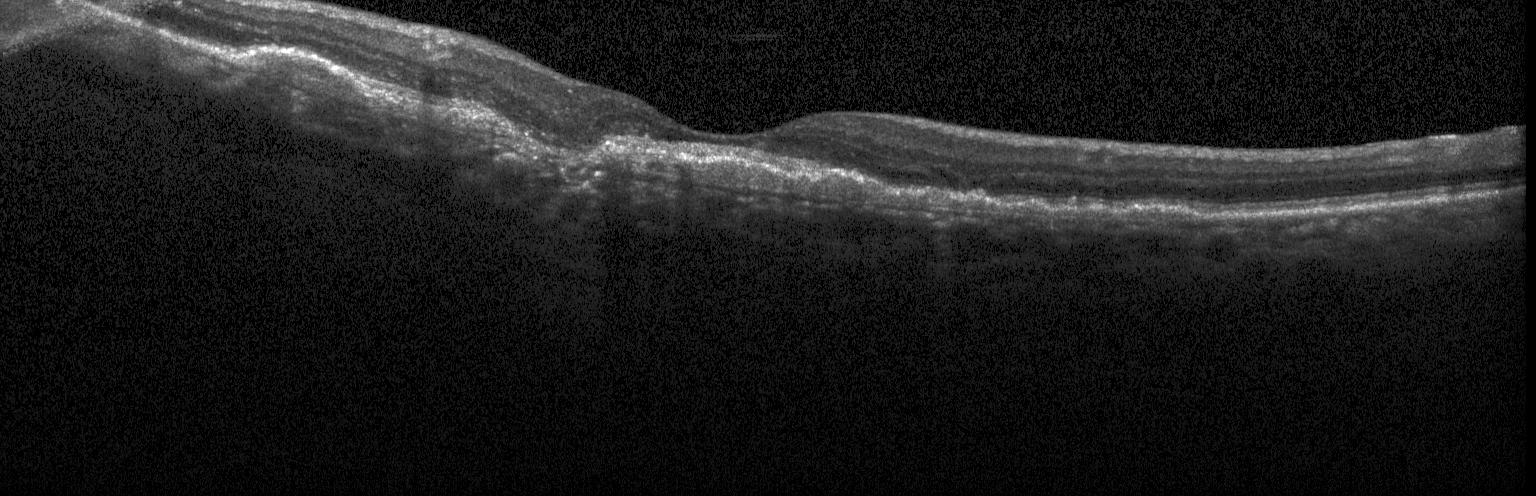

Macular scan · Heidelberg Spectralis · SD-OCT · optical coherence tomography B-scan.
A choroidal neovascular membrane.